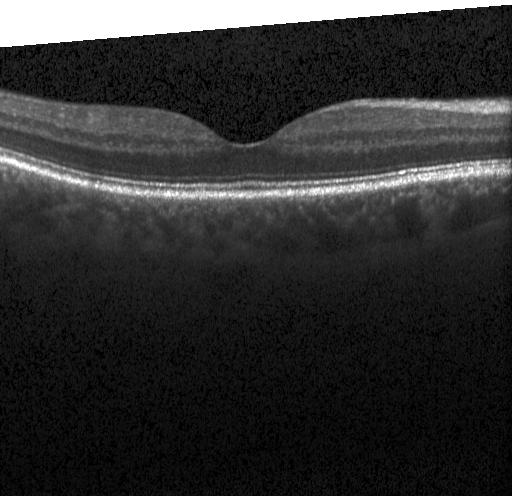 Retinal OCT cross-section, spectral-domain optical coherence tomography, Heidelberg Spectralis
This B-scan demonstrates no evidence of choroidal neovascularization, diabetic macular edema, or drusen.